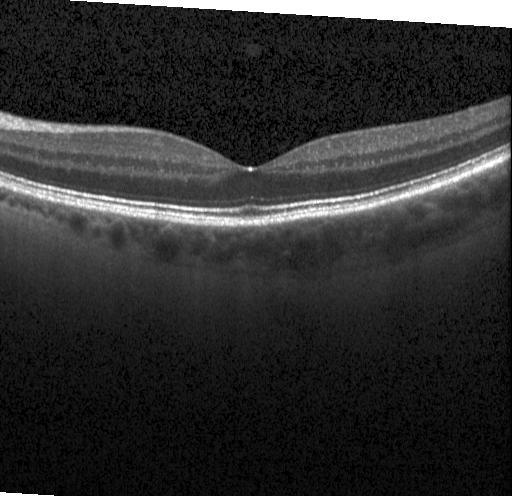
Dx: neither CNV, DME, nor drusen.